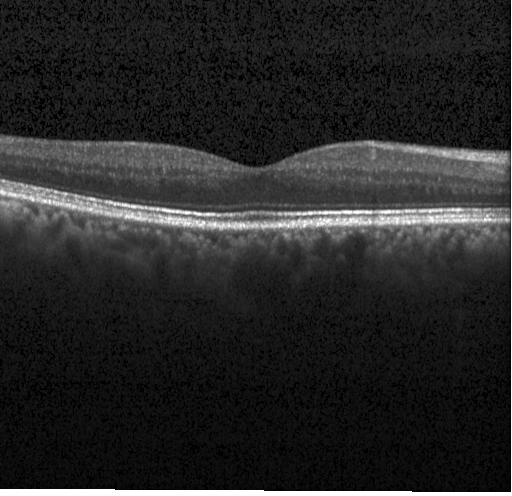
Acquired on a Heidelberg Spectralis, retinal OCT cross-section, centered on the fovea, spectral-domain OCT.
OCT finding: no evidence of choroidal neovascularization, diabetic macular edema, or drusen.